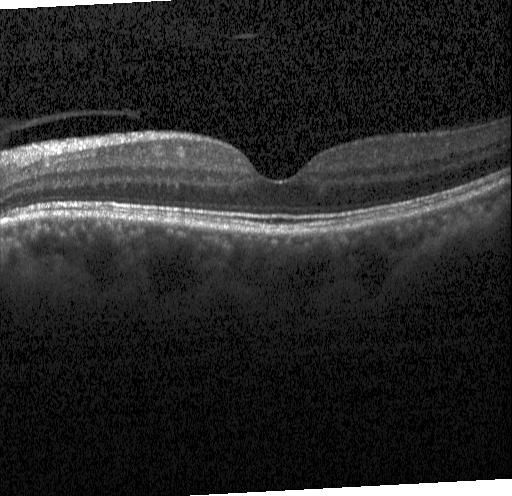

Through the macula. Spectral-domain optical coherence tomography. Retinal OCT cross-section. OCT finding: no evidence of choroidal neovascularization, diabetic macular edema, or drusen.